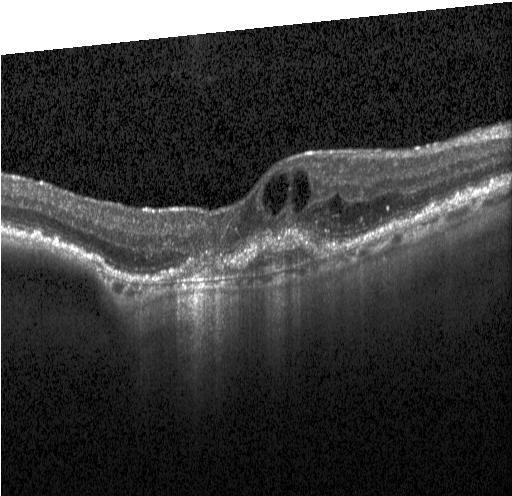

The scan shows CNV.